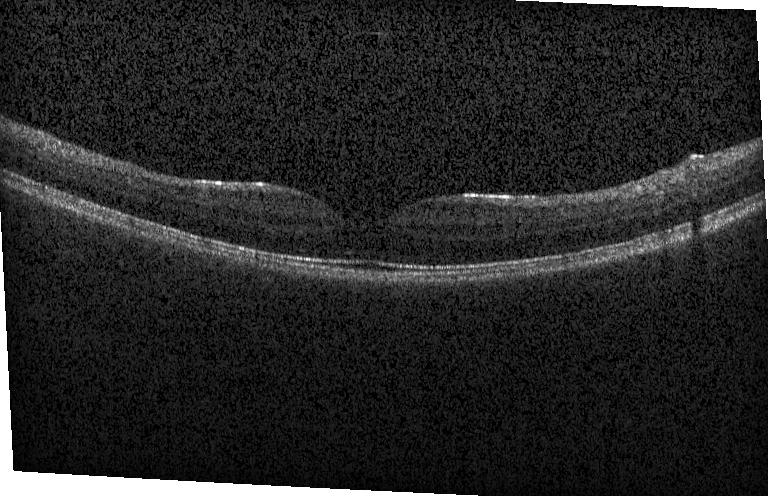 OCT B-scan. Macular scan. Heidelberg Spectralis OCT system. Spectral-domain optical coherence tomography.
No CNV, no DME, and no drusen.